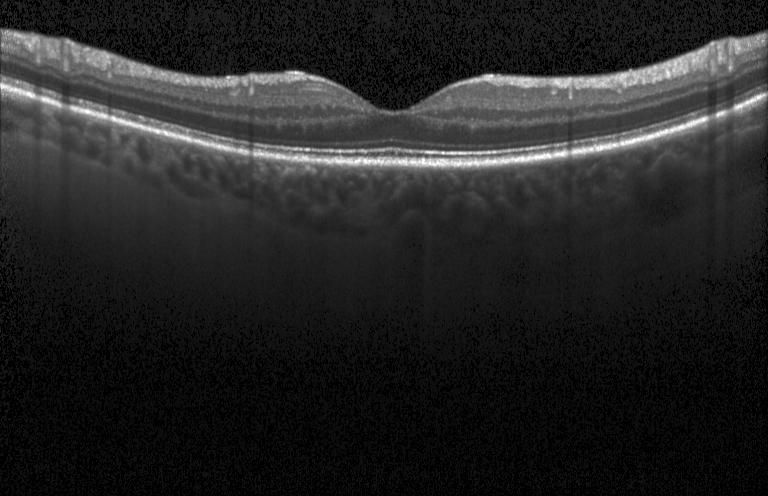

OCT line scan — No evidence of choroidal neovascularization, diabetic macular edema, or drusen.